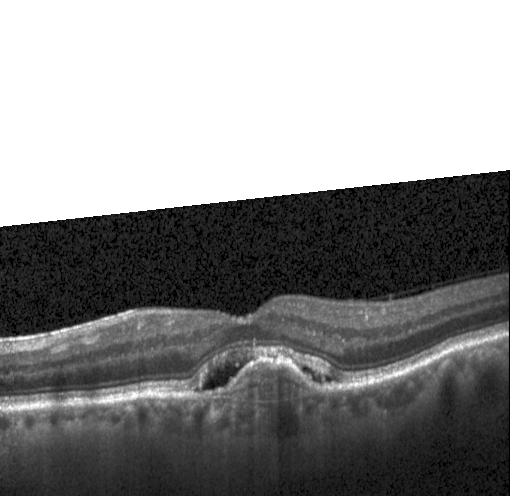
Optical coherence tomography B-scan · macular scan — Finding: CNV.